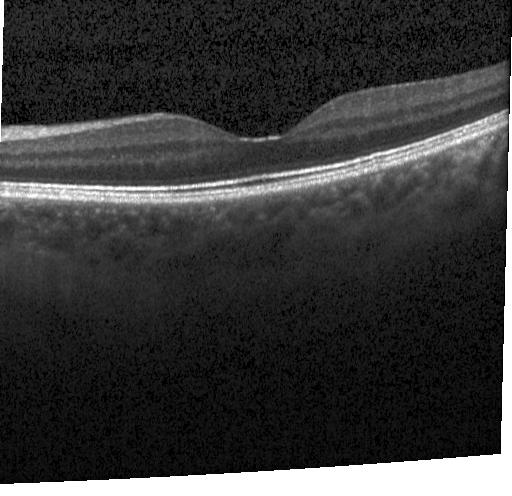

SD-OCT, optical coherence tomography B-scan
This B-scan demonstrates neither CNV, DME, nor drusen.